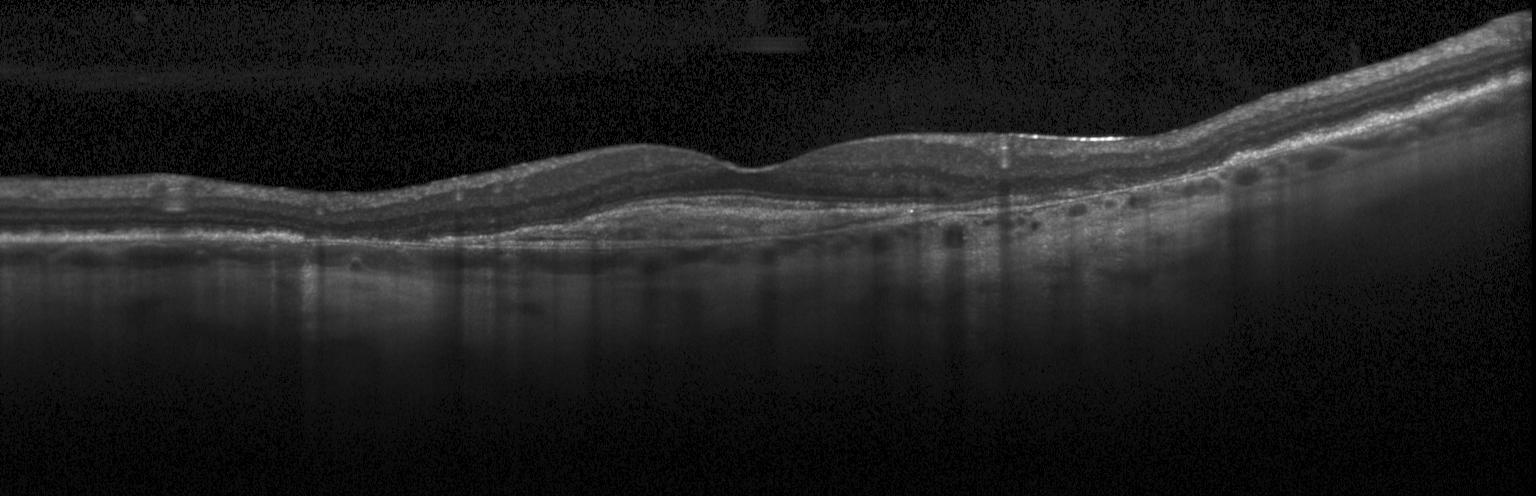
Optical coherence tomography scan
Dx: choroidal neovascularization.